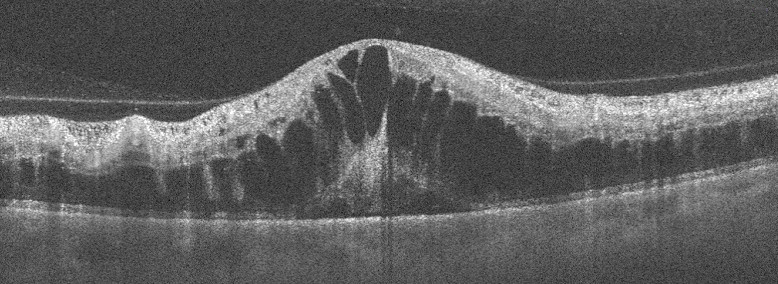

Retinal OCT B-scan · through the macula. Assessment: RVO.